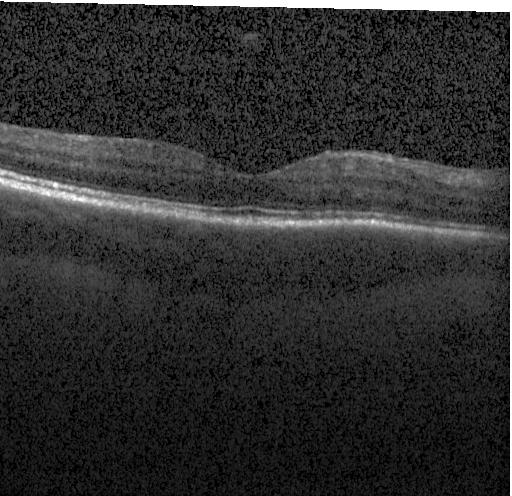 OCT B-scan showing no choroidal neovascularization, no diabetic macular edema, and no drusen.